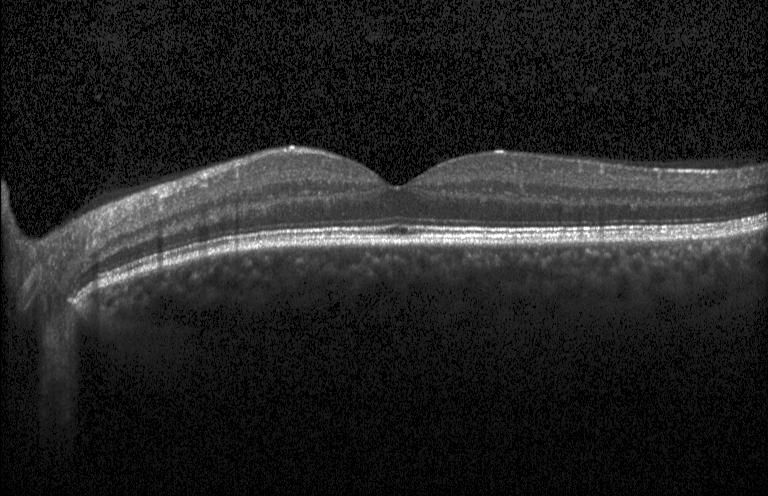

Optical coherence tomography scan. The scan shows no choroidal neovascularization, no diabetic macular edema, and no drusen.